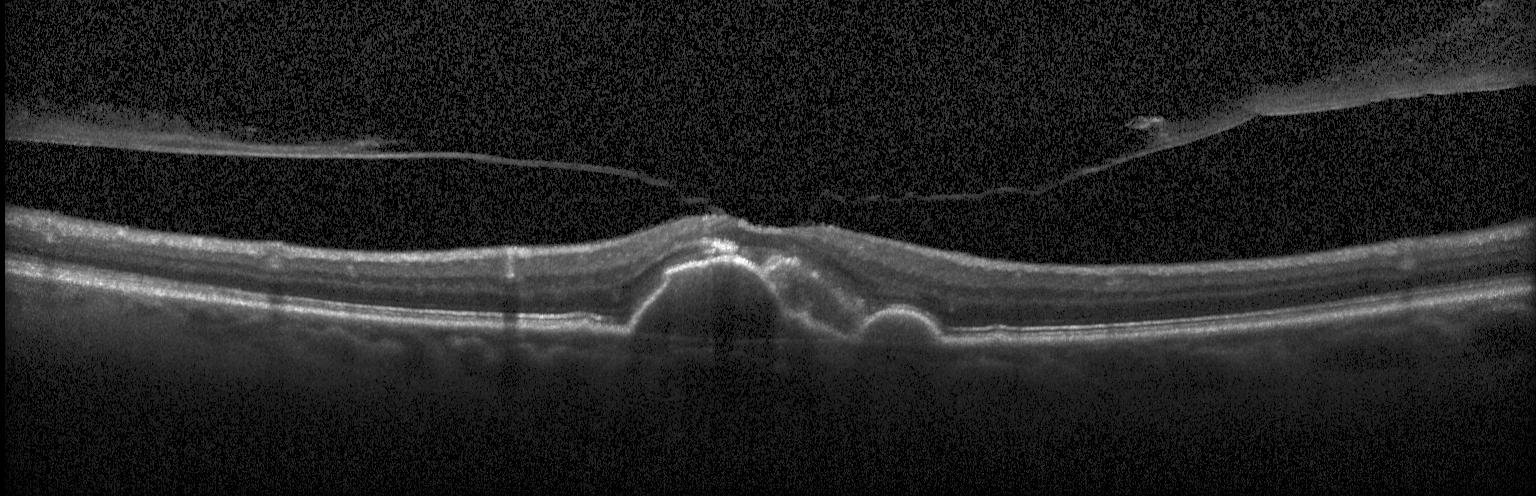
OCT scan showing choroidal neovascularization (CNV).